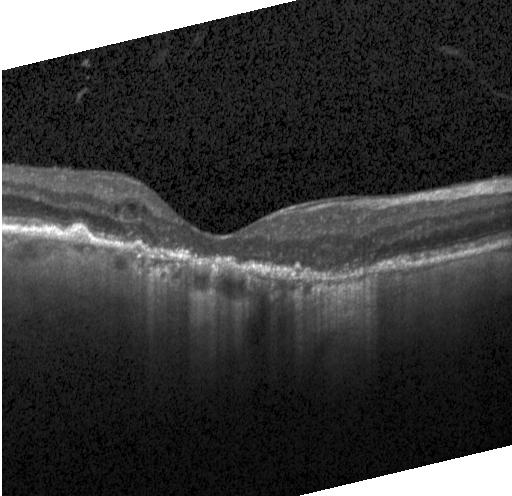
The scan shows CNV.